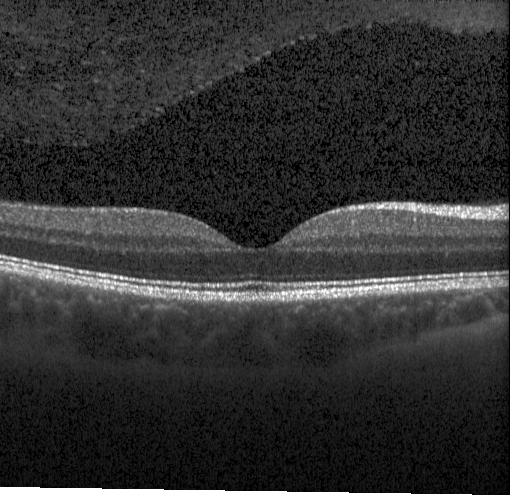

OCT finding: no choroidal neovascularization, no diabetic macular edema, and no drusen.